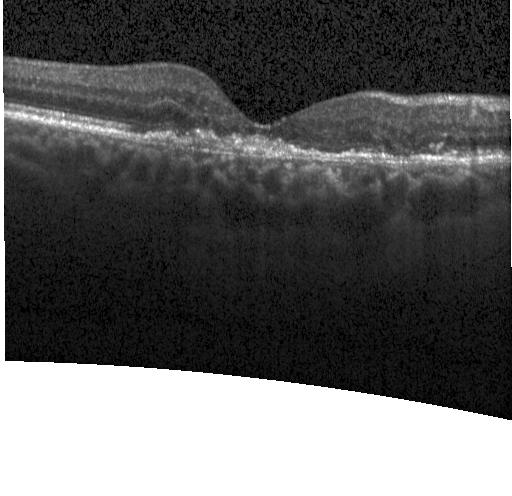
Through the macula · optical coherence tomography B-scan · Heidelberg Spectralis.
Assessment: CNV.